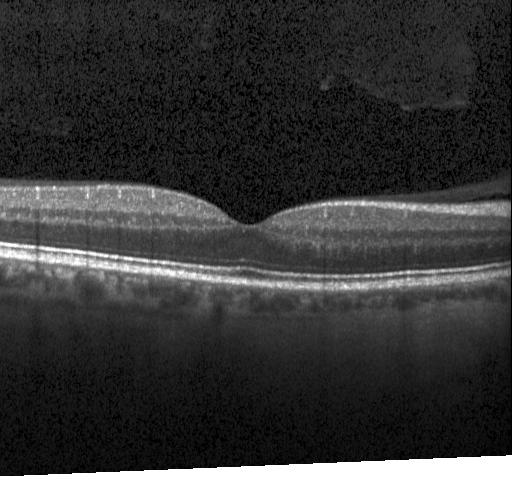 OCT B-scan, spectral-domain OCT.
Impression: neither choroidal neovascularization, diabetic macular edema, nor drusen.